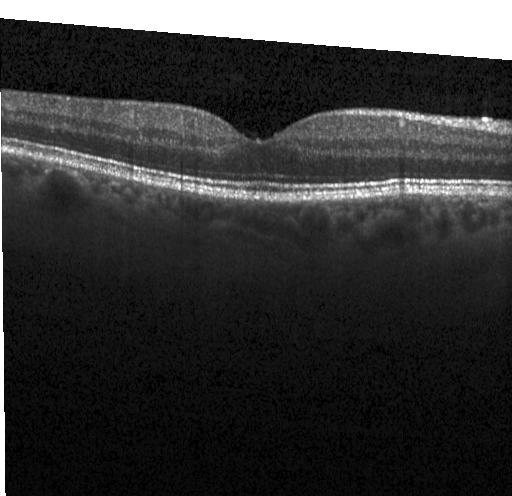

Through the macula. Instrument: Heidelberg Spectralis. Optical coherence tomography scan — Impression: no choroidal neovascularization, no diabetic macular edema, and no drusen.